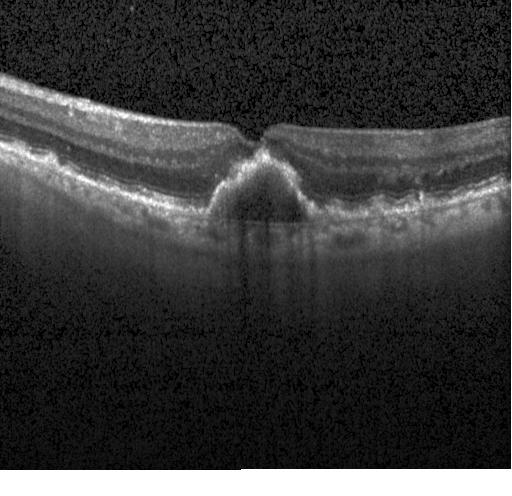
Retinal OCT B-scan, acquired on a Heidelberg Spectralis.
Impression: a choroidal neovascular membrane.